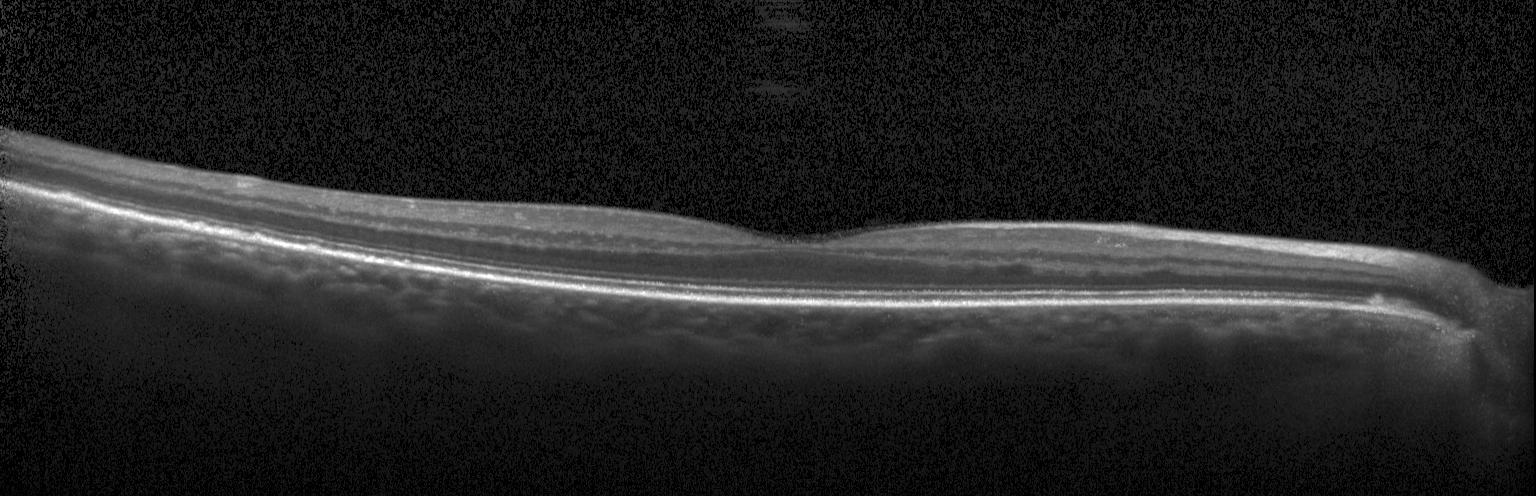 Acquired on a Heidelberg Spectralis. SD-OCT. OCT line scan — Finding: no evidence of choroidal neovascularization, diabetic macular edema, or drusen.